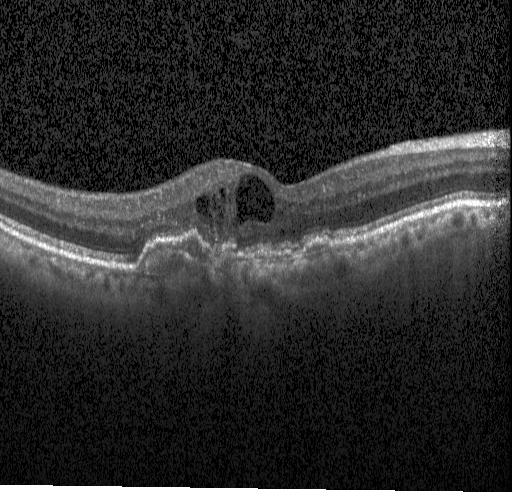

Macular OCT demonstrating choroidal neovascularization.